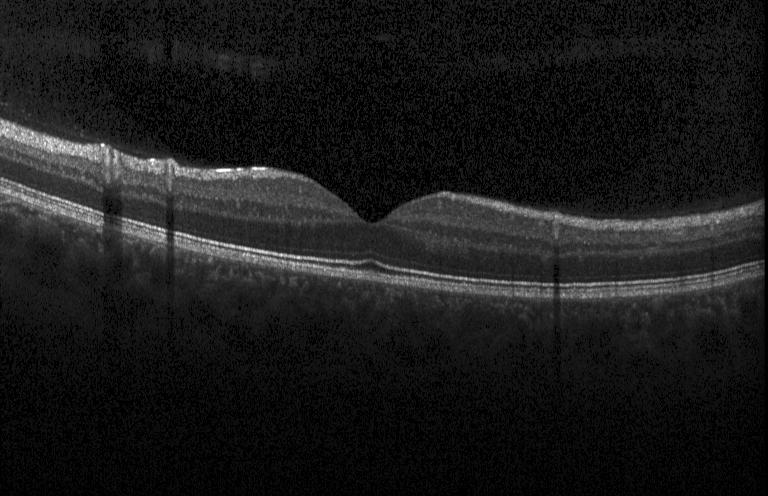
Centered on the fovea. Spectral-domain optical coherence tomography. OCT line scan. Acquired on a Heidelberg Spectralis — The scan shows no CNV, DME, or drusen.